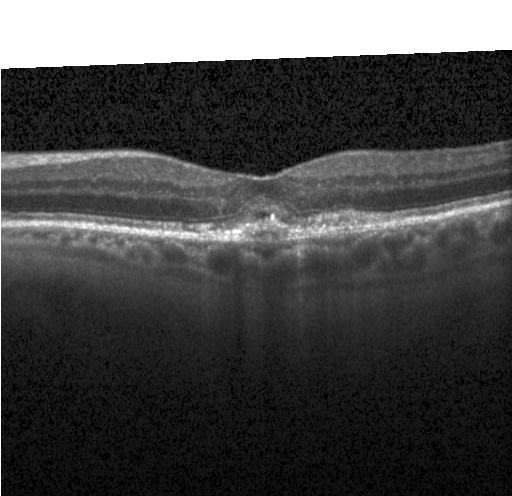
Retinal OCT cross-section
Finding: a choroidal neovascular membrane.